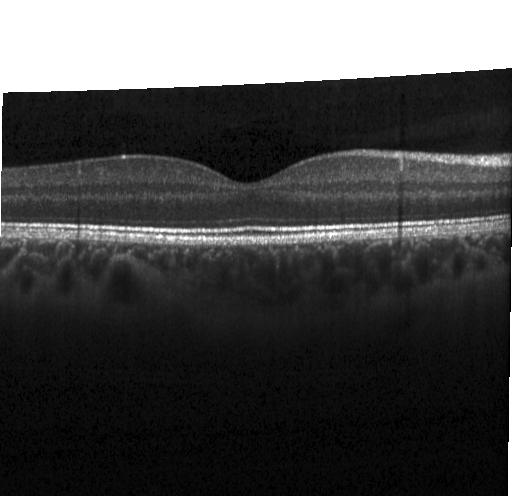

OCT line scan · through the macula · Heidelberg Spectralis OCT system — Finding: no choroidal neovascularization, diabetic macular edema, or drusen.